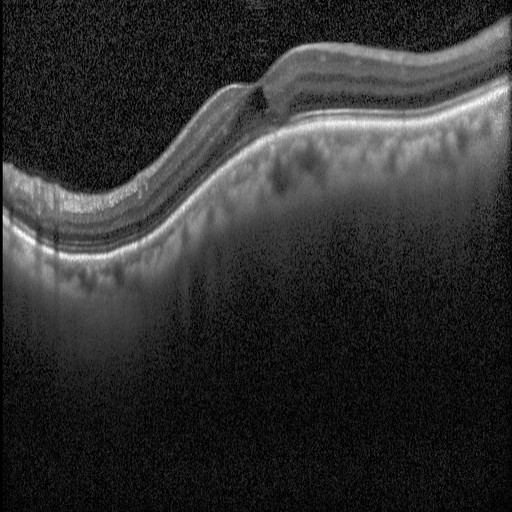

OCT scan showing diabetic macular edema.